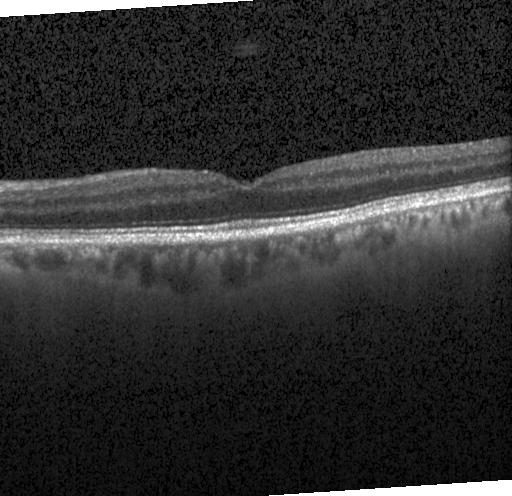
Heidelberg Spectralis OCT system, retinal OCT cross-section. Diagnosis: no evidence of CNV, DME, or drusen.